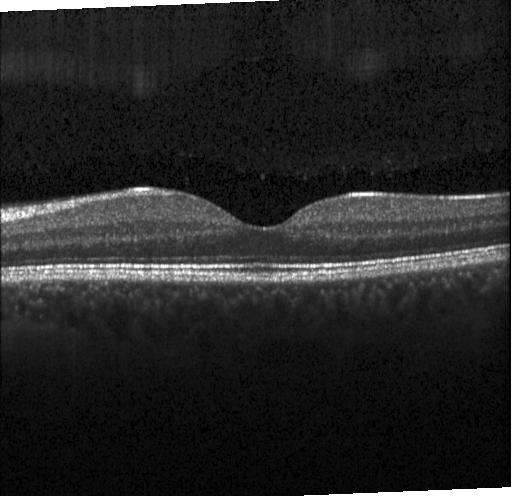 Macular scan, SD-OCT, optical coherence tomography B-scan, Heidelberg Spectralis
Finding: neither choroidal neovascularization, diabetic macular edema, nor drusen.